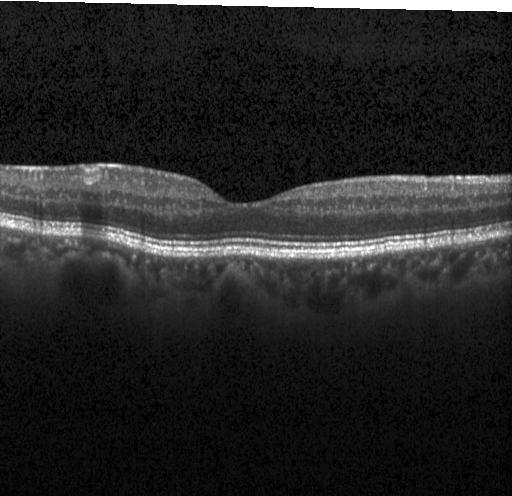

Impression: no CNV, no DME, and no drusen.